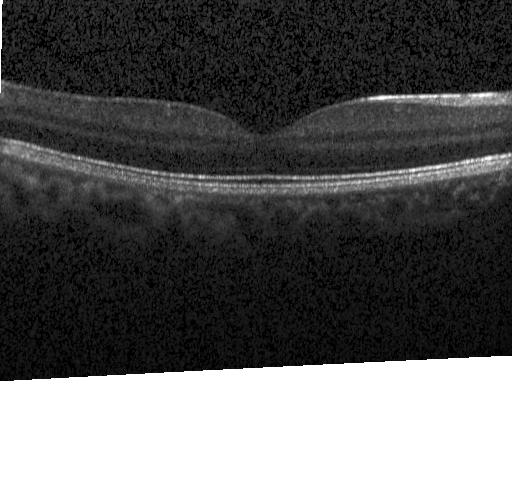
Fovea-centered · spectral-domain OCT · optical coherence tomography scan · instrument: Heidelberg Spectralis.
Neither CNV, DME, nor drusen.